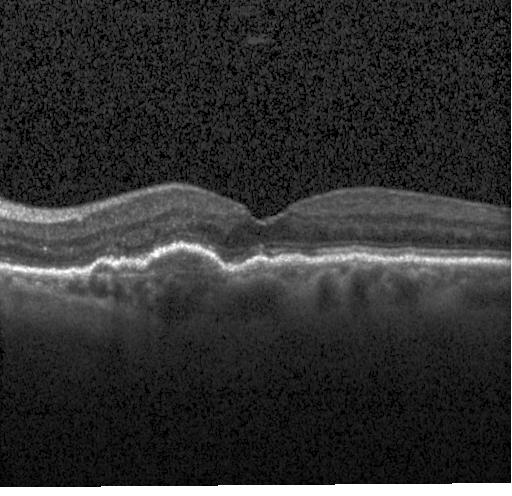 Retinal OCT B-scan — Assessment: a choroidal neovascular membrane.